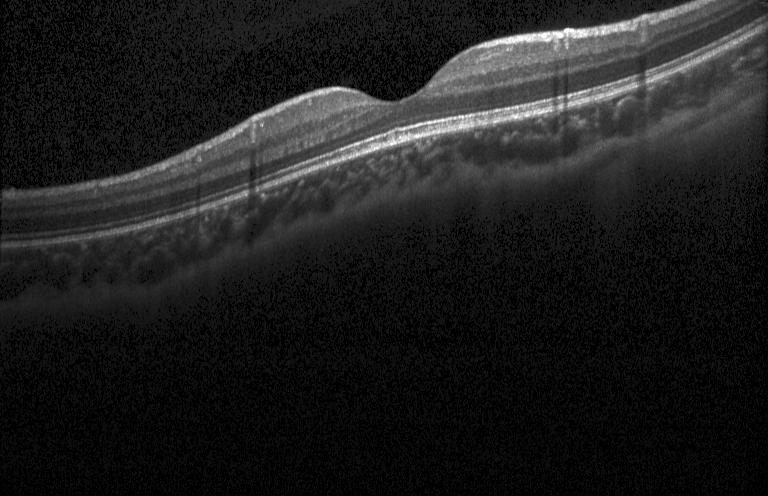 Acquired on a Heidelberg Spectralis · SD-OCT · retinal OCT B-scan
Dx: neither choroidal neovascularization, diabetic macular edema, nor drusen.